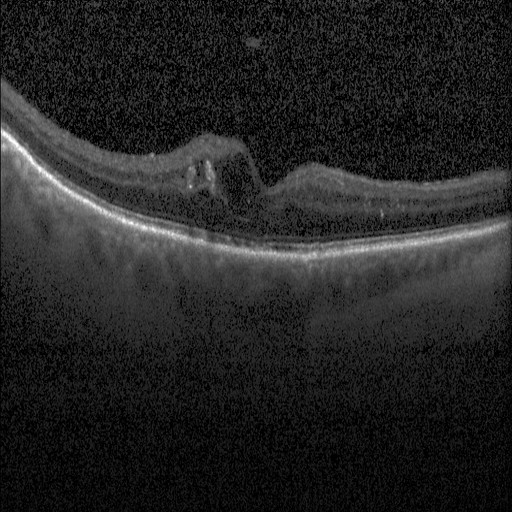
OCT line scan. Instrument: Heidelberg Spectralis. Impression: diabetic macular edema (DME).